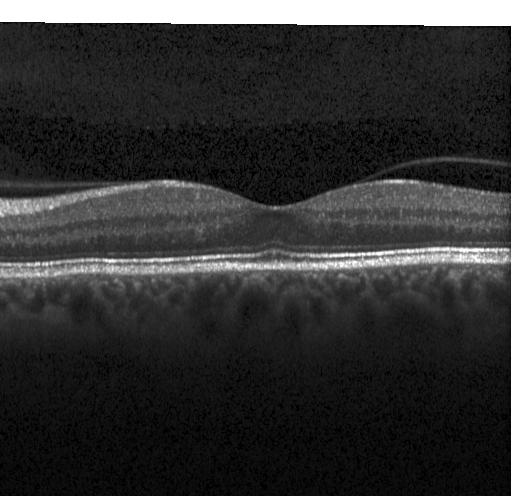
Optical coherence tomography scan; centered on the fovea; spectral-domain OCT; Heidelberg Spectralis OCT system — No CNV, no DME, and no drusen.